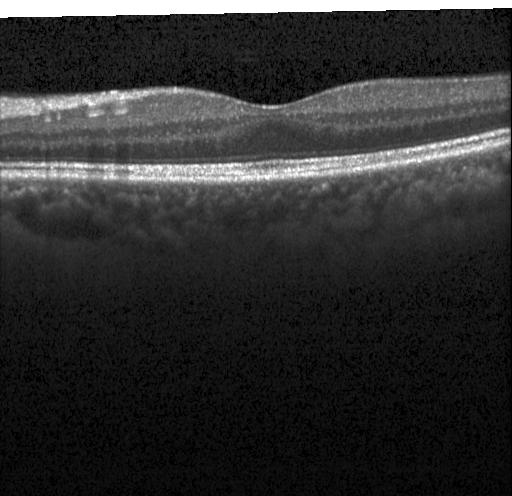 Macular OCT: neither CNV, DME, nor drusen.